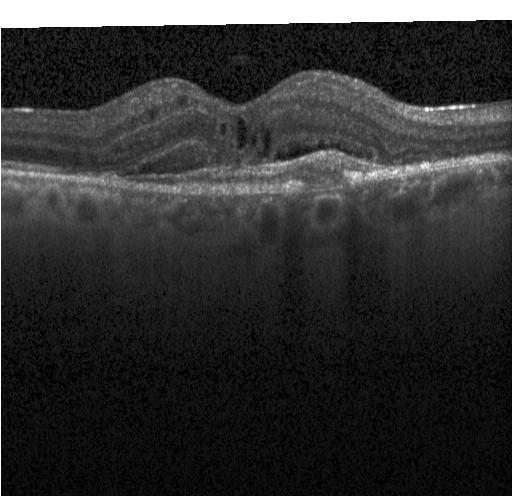 OCT line scan, spectral-domain optical coherence tomography, acquired on a Heidelberg Spectralis. A choroidal neovascular membrane.